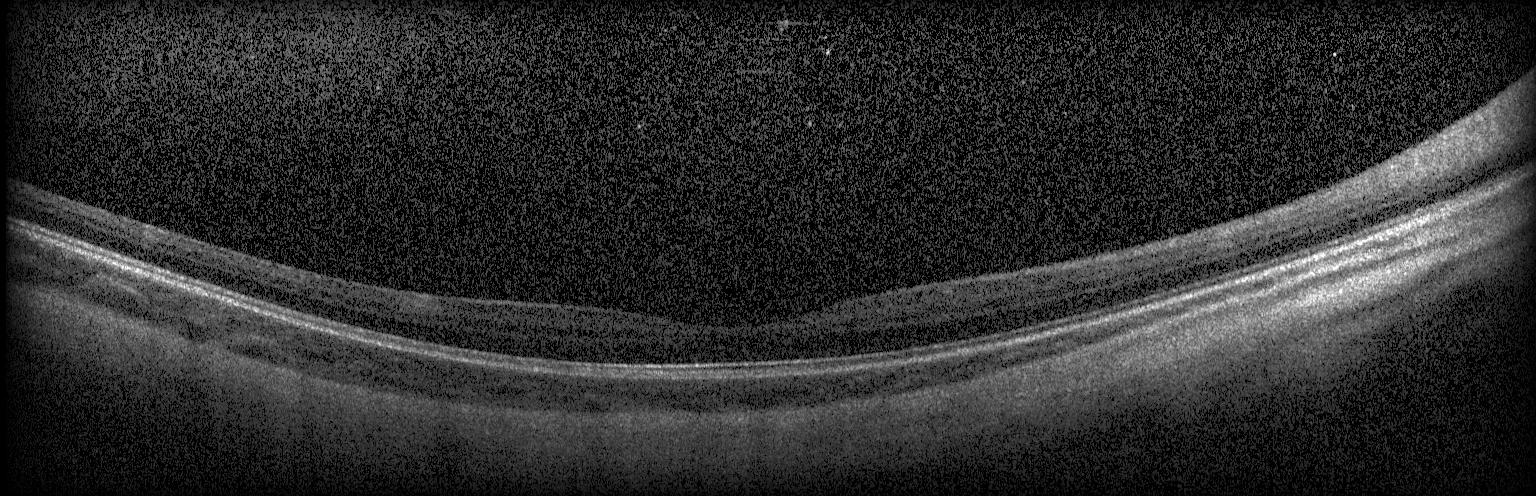 SD-OCT; macular scan; Heidelberg Spectralis OCT system; retinal OCT B-scan
Assessment: no evidence of CNV, DME, or drusen.